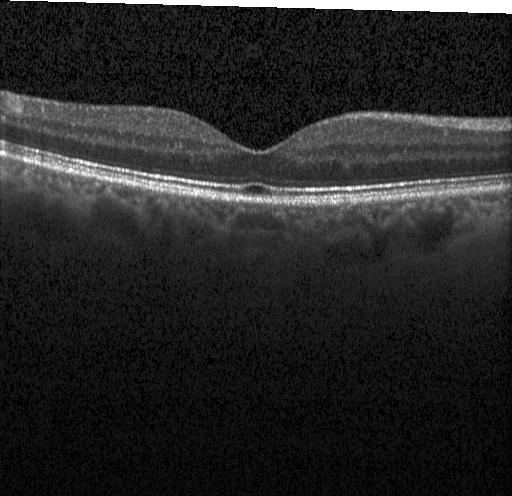 Macular OCT: neither choroidal neovascularization, diabetic macular edema, nor drusen.